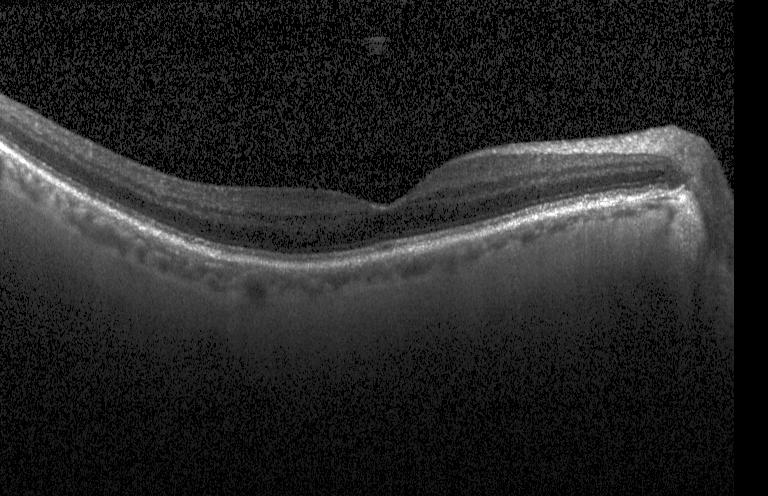
Finding: neither choroidal neovascularization, diabetic macular edema, nor drusen.